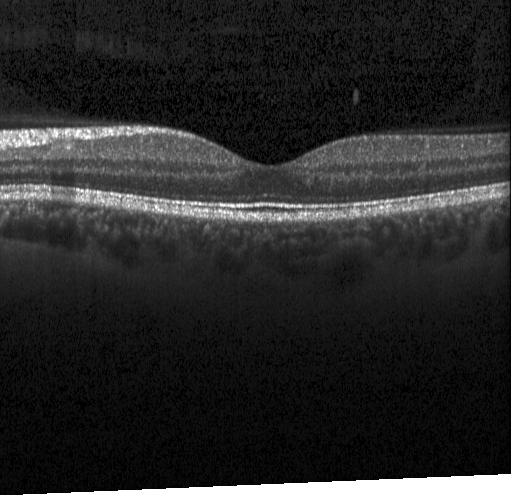

Optical coherence tomography B-scan.
Assessment: no CNV, DME, or drusen.